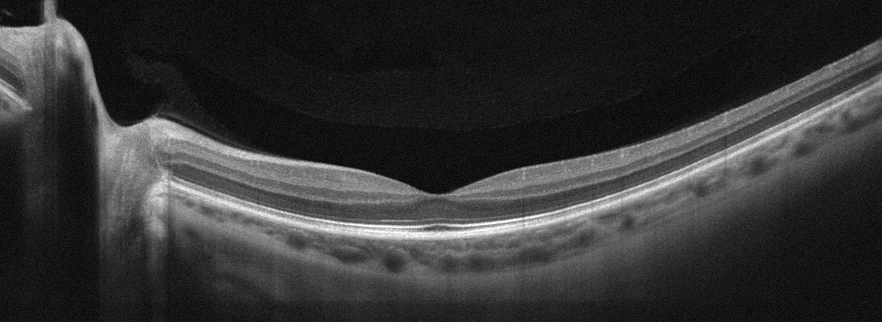 OS · retinal OCT cross-section. Impression: no evidence of AMD, DME, ERM, RAO, RVO, or VID.